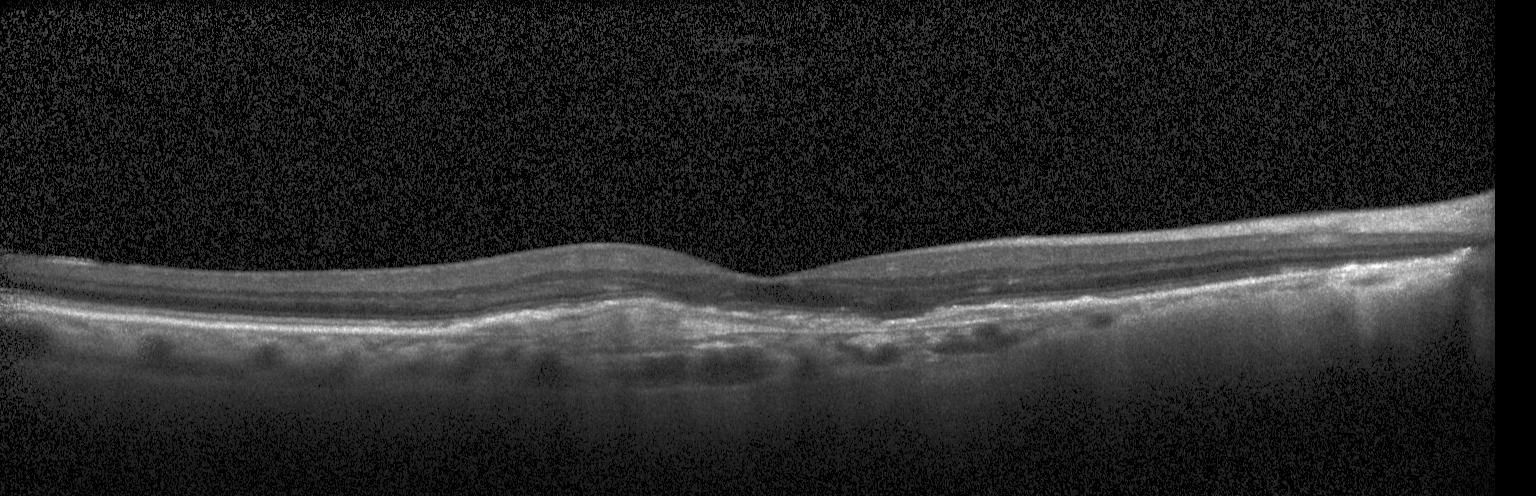

Optical coherence tomography scan · Heidelberg Spectralis OCT system — Finding: a choroidal neovascular membrane.